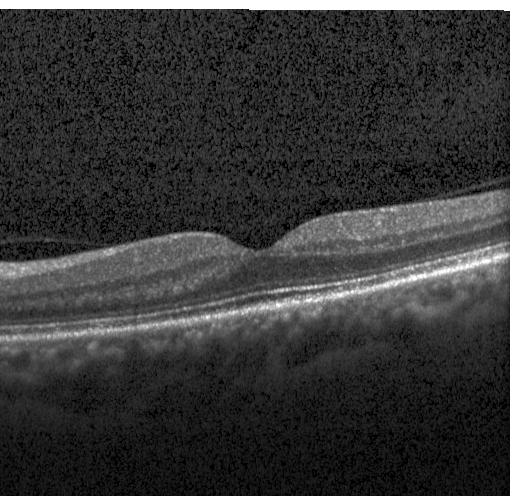
Retinal OCT B-scan; spectral-domain optical coherence tomography; Heidelberg Spectralis OCT system; through the macula
Impression: no choroidal neovascularization, diabetic macular edema, or drusen.